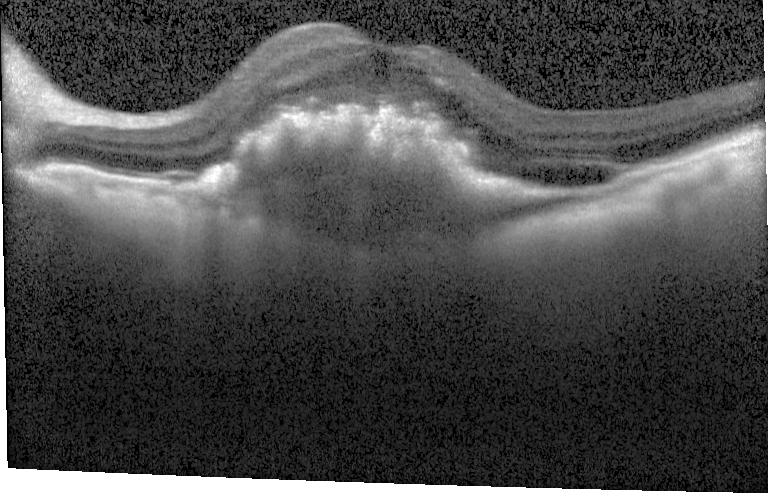 Optical coherence tomography B-scan — OCT finding: CNV.